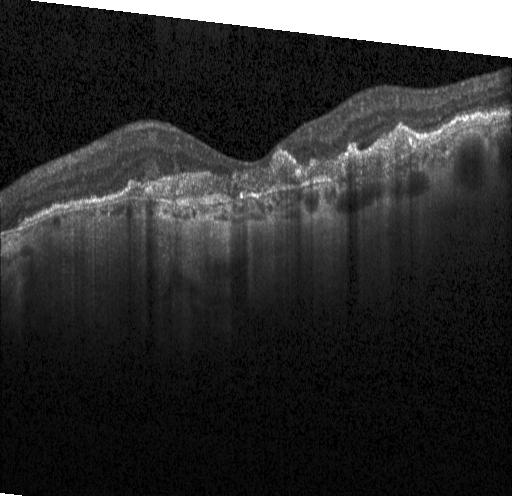 Diagnosis: choroidal neovascularization (CNV).